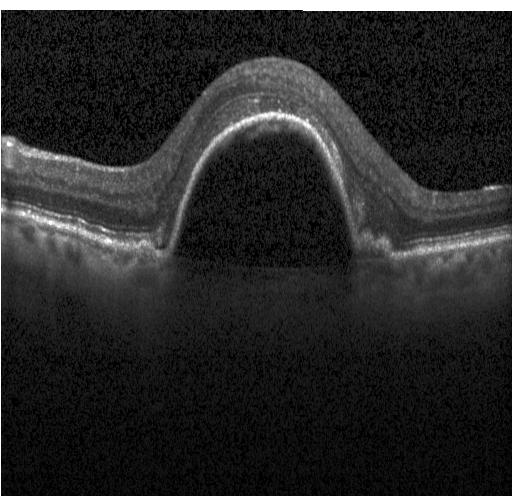 OCT B-scan. Diagnosis: choroidal neovascularization (CNV).